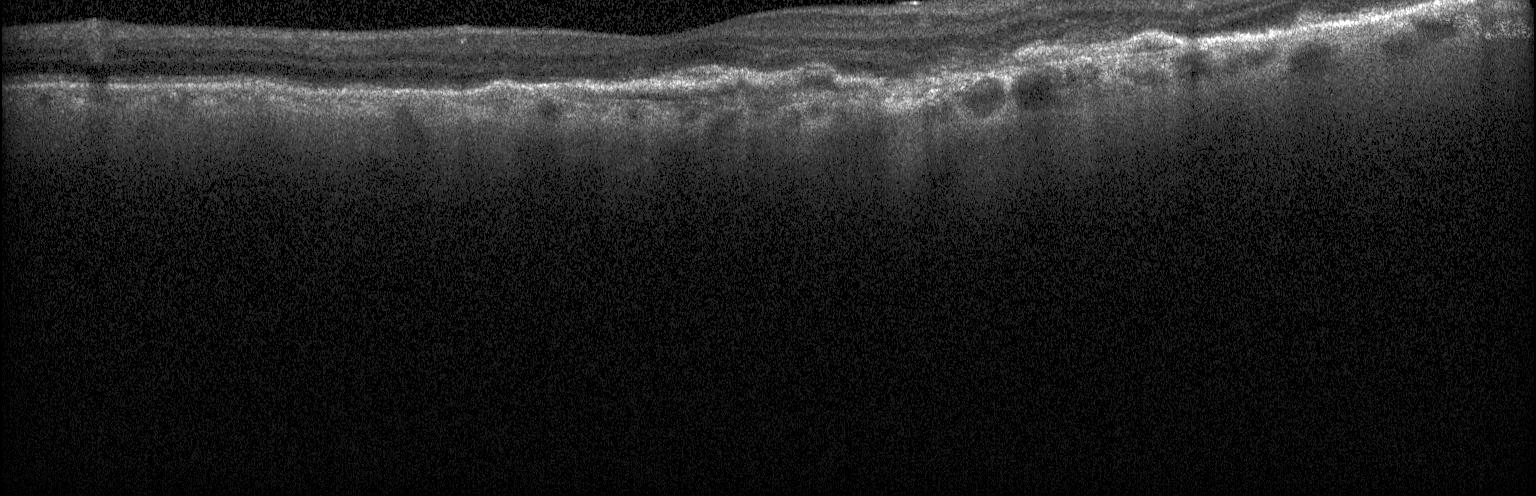

Optical coherence tomography B-scan. Acquired on a Heidelberg Spectralis. Spectral-domain optical coherence tomography. Macular scan
Dx: CNV.